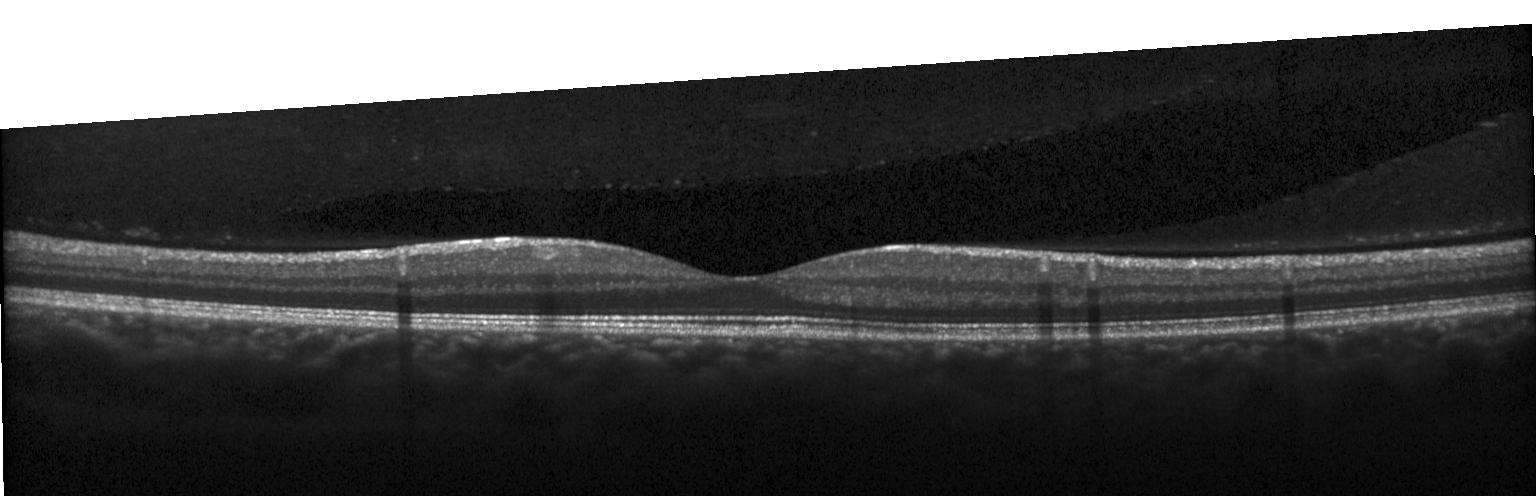 Impression: no choroidal neovascularization, diabetic macular edema, or drusen.